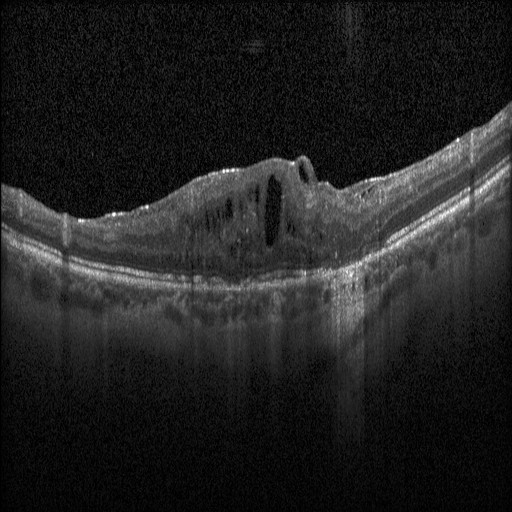
Spectral-domain OCT B-scan: DME.